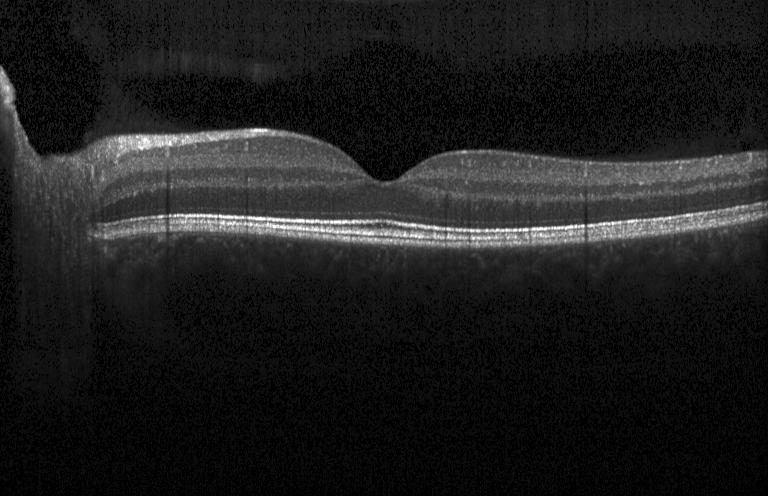 Heidelberg Spectralis · retinal OCT B-scan · spectral-domain optical coherence tomography · centered on the fovea.
Dx: no evidence of choroidal neovascularization, diabetic macular edema, or drusen.